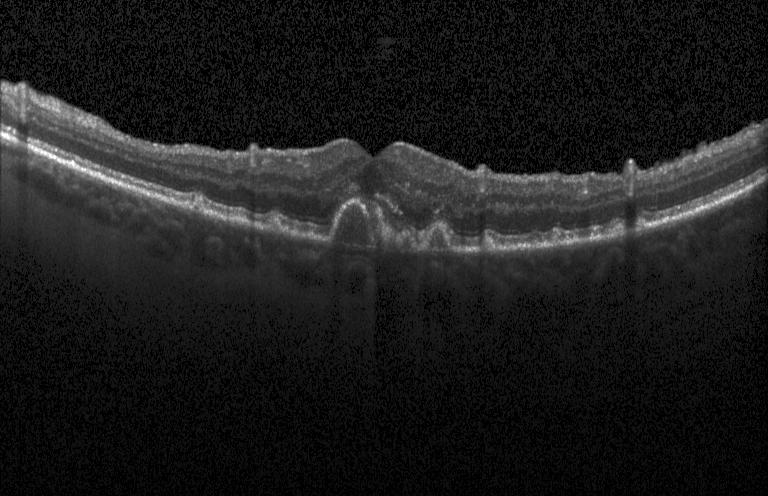
Retinal OCT B-scan, centered on the fovea, instrument: Heidelberg Spectralis
This B-scan demonstrates sub-RPE drusenoid deposits.